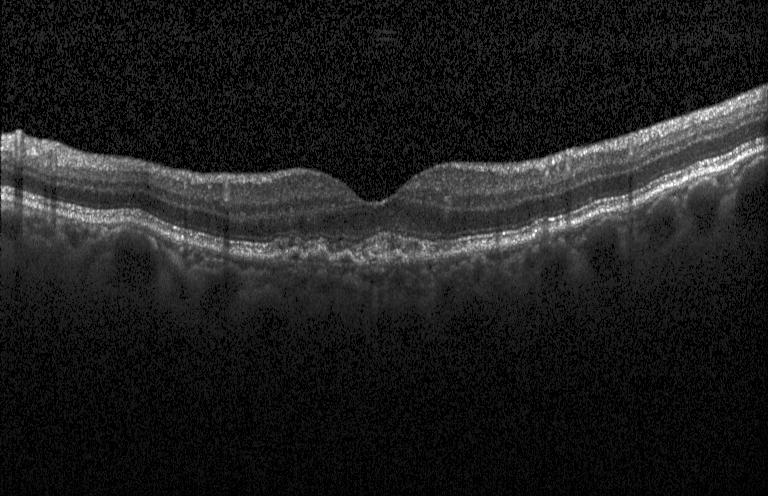
Assessment: a choroidal neovascular membrane.